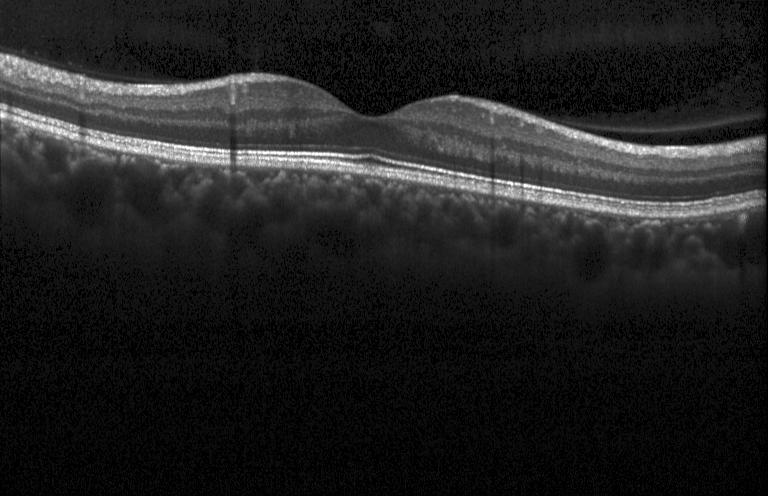
Retinal OCT cross-section. Dx: neither choroidal neovascularization, diabetic macular edema, nor drusen.